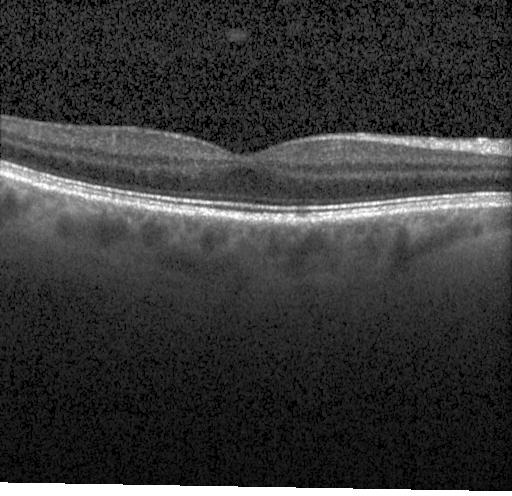
Diagnosis: no CNV, no DME, and no drusen.